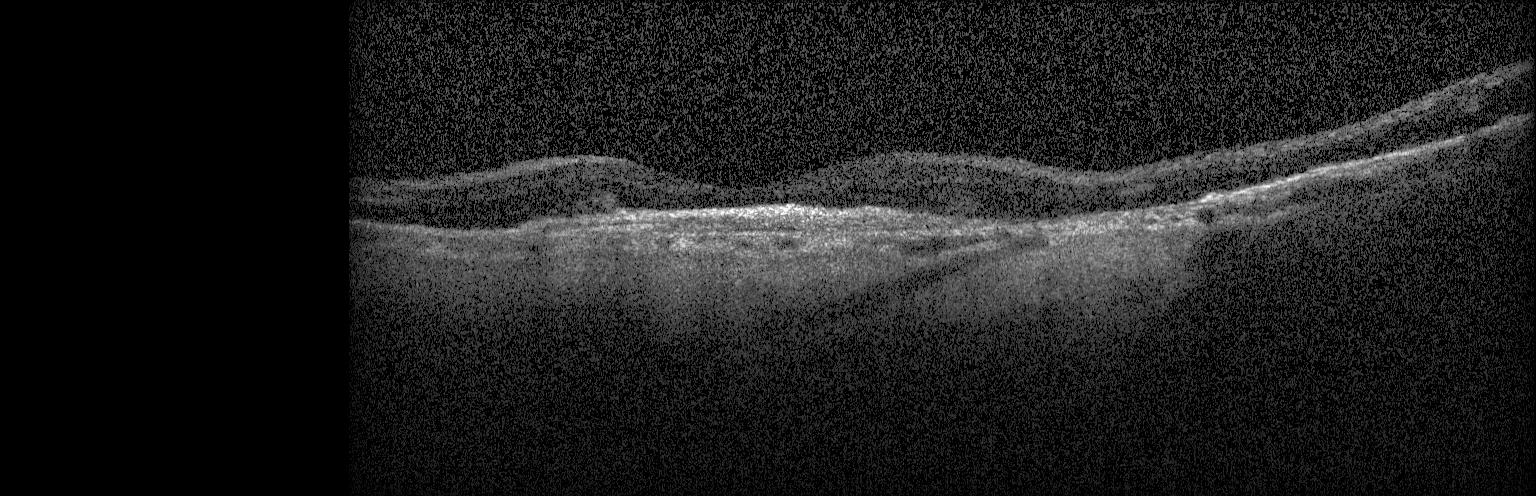 Instrument: Heidelberg Spectralis · spectral-domain OCT · fovea-centered · OCT B-scan.
Impression: CNV.